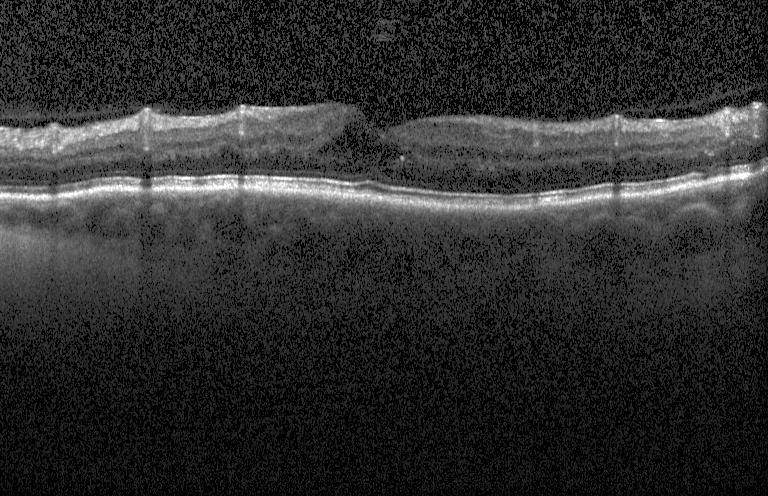

Spectral-domain OCT. OCT line scan.
OCT finding: diabetic macular edema (DME).